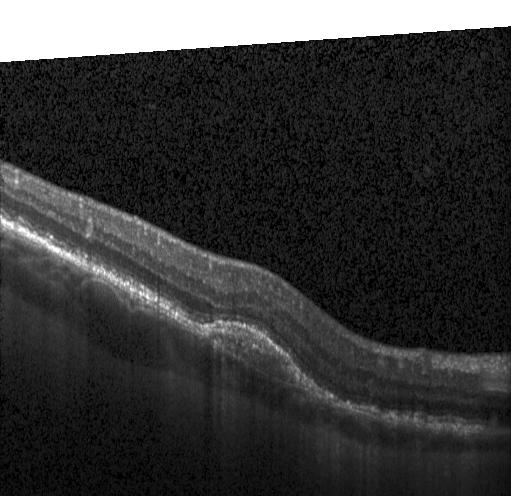 OCT B-scan, SD-OCT.
The scan shows a choroidal neovascular membrane.